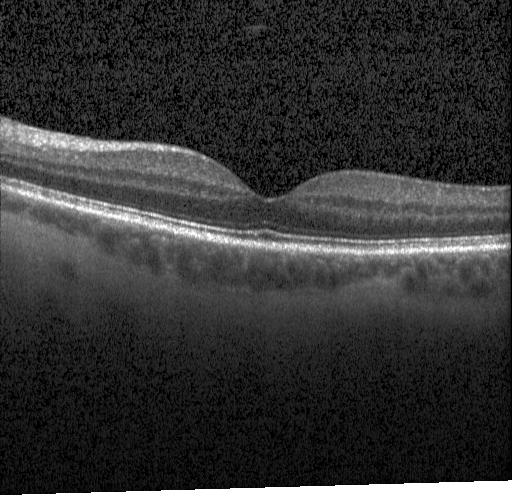
Optical coherence tomography B-scan. Finding: no CNV, no DME, and no drusen.